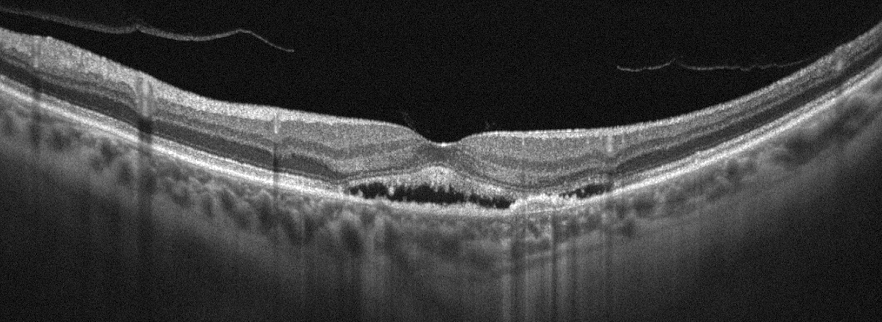
Macular OCT: age-related macular degeneration.